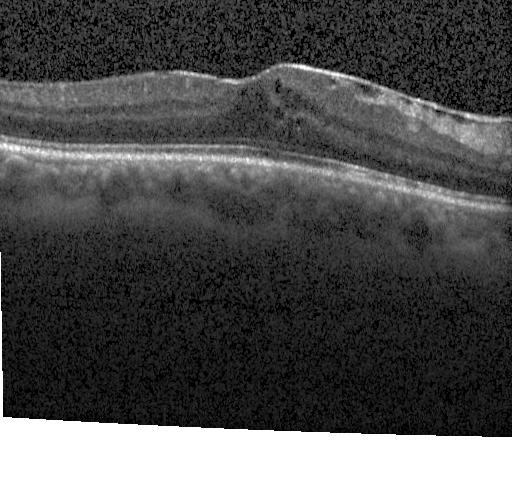 Retinal OCT B-scan; spectral-domain OCT; macular scan; acquired on a Heidelberg Spectralis — Impression: diabetic macular edema (DME).